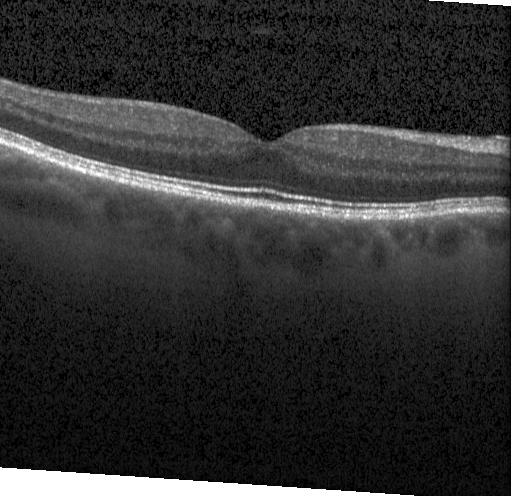

SD-OCT, fovea-centered, instrument: Heidelberg Spectralis, retinal OCT B-scan. Impression: neither CNV, DME, nor drusen.